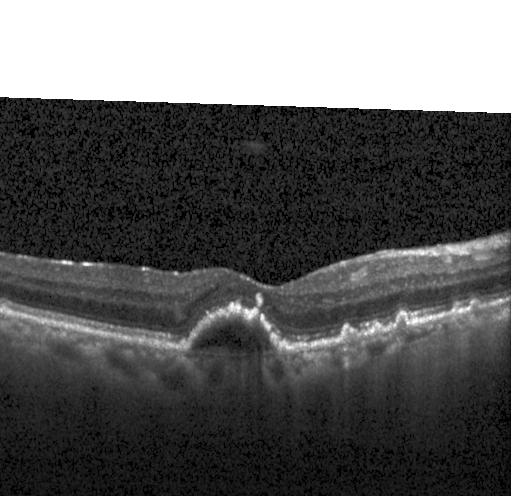
Diagnosis: CNV.